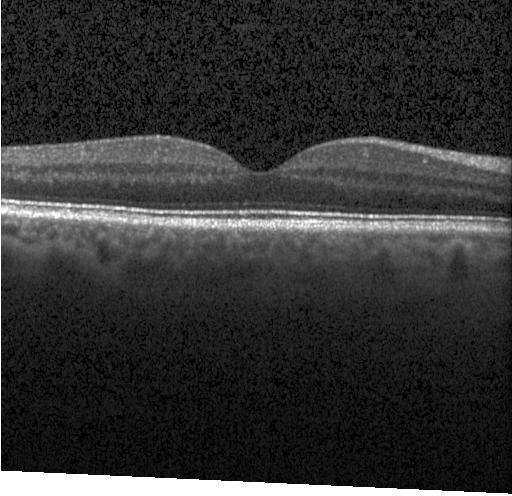
Macular OCT demonstrating no choroidal neovascularization, diabetic macular edema, or drusen.